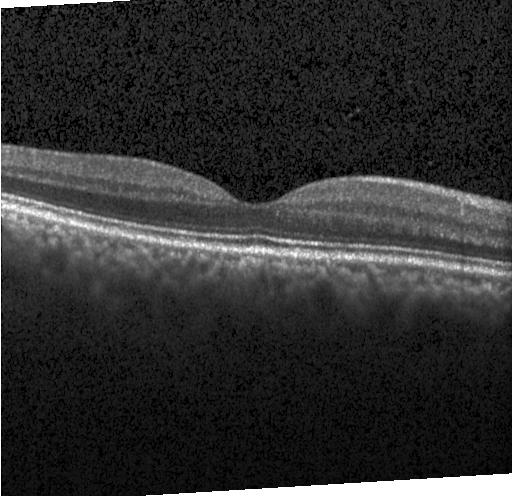 OCT line scan.
The scan shows no evidence of CNV, DME, or drusen.